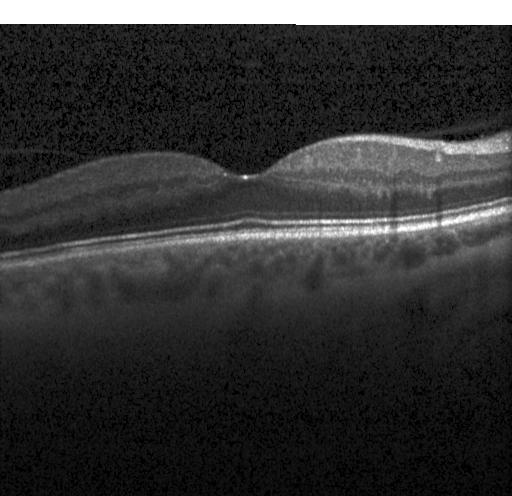

Impression: no choroidal neovascularization, diabetic macular edema, or drusen.